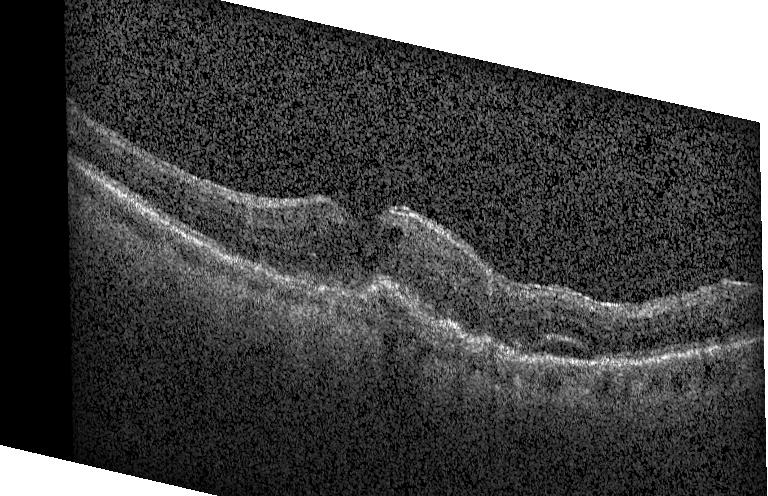

Retinal OCT cross-section
Macular OCT: a choroidal neovascular membrane.